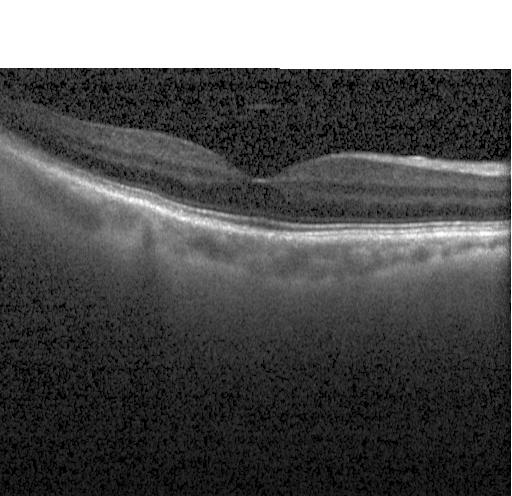
OCT line scan. No choroidal neovascularization, diabetic macular edema, or drusen.